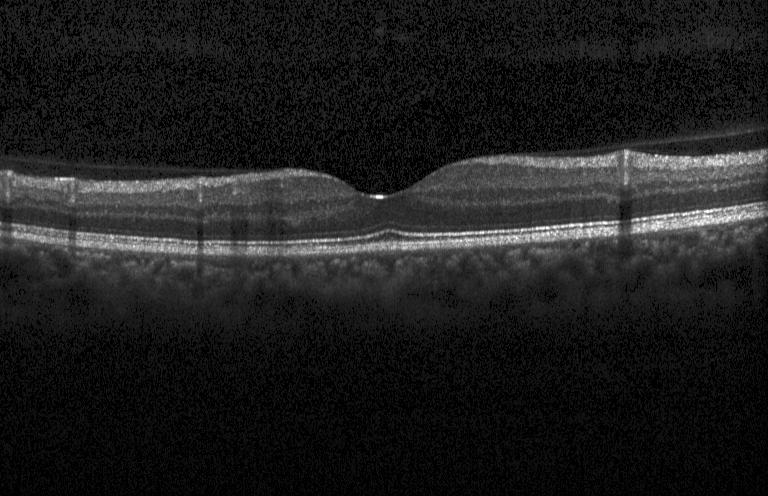 OCT finding: no evidence of choroidal neovascularization, diabetic macular edema, or drusen.